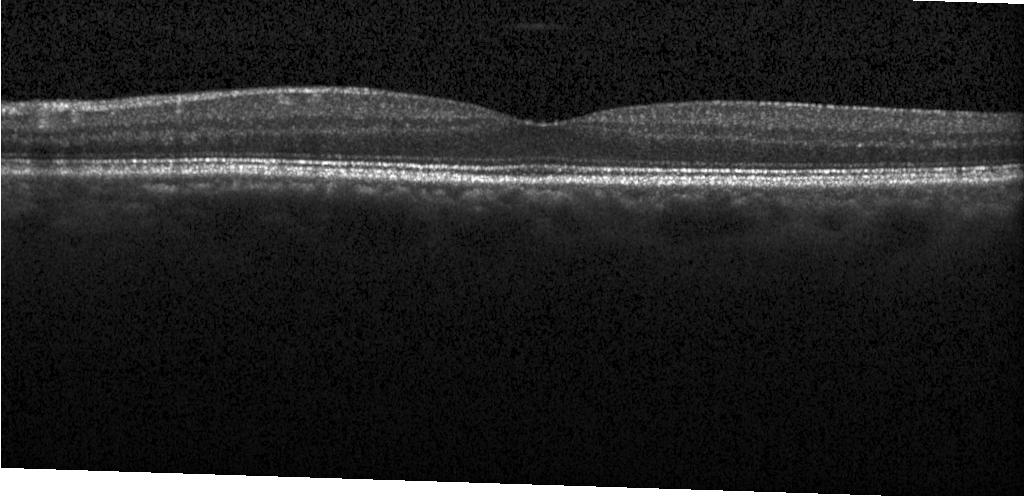

Instrument: Heidelberg Spectralis. Optical coherence tomography B-scan. Through the macula — Dx: neither CNV, DME, nor drusen.